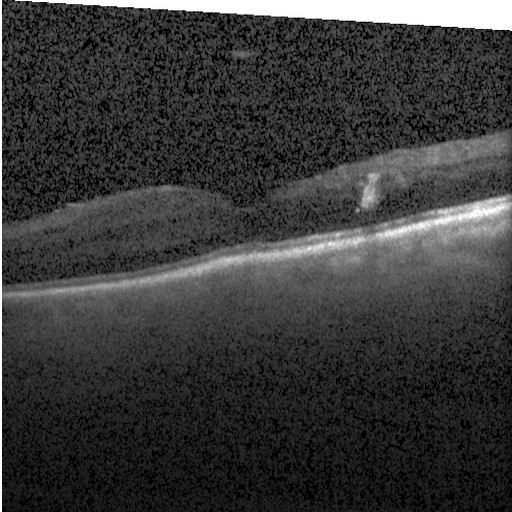
Instrument: Heidelberg Spectralis; OCT line scan.
Assessment: DME.